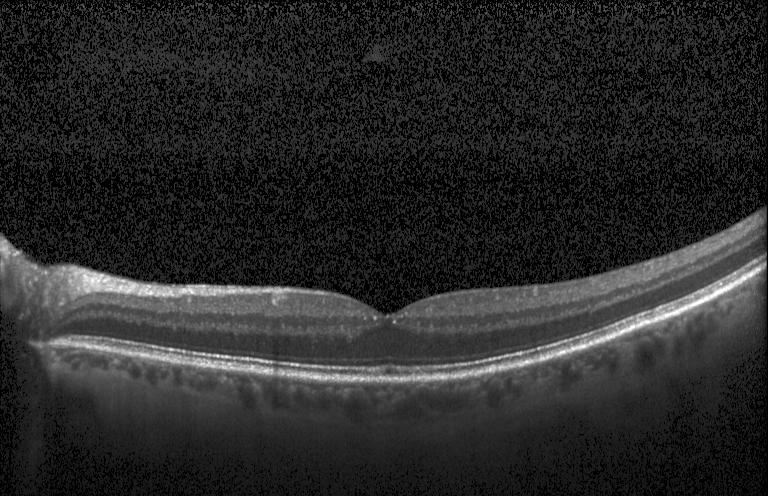 Retinal OCT B-scan.
Finding: no evidence of CNV, DME, or drusen.